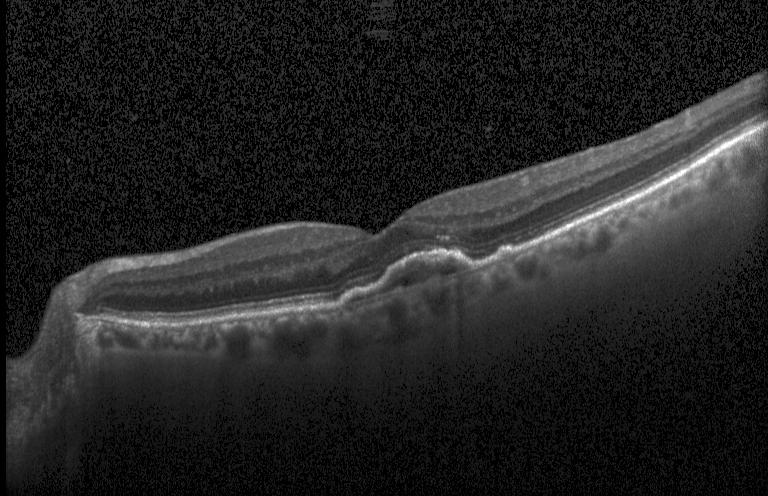

Macular OCT demonstrating CNV.